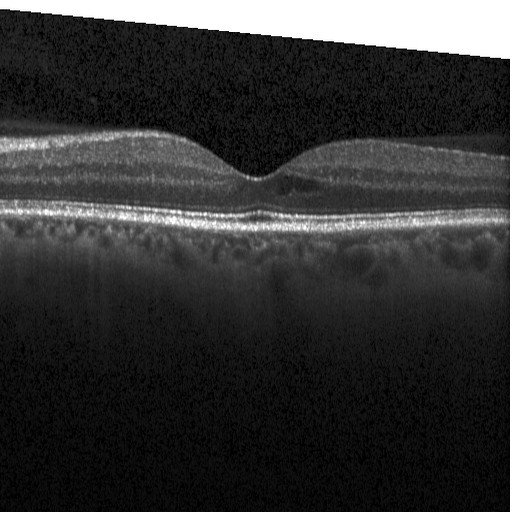 Diagnosis: diabetic macular edema.